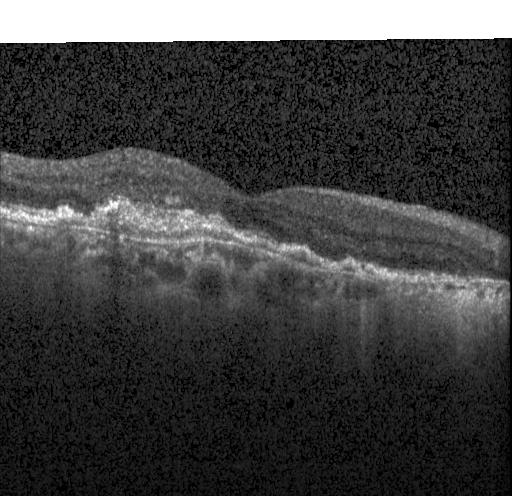 OCT B-scan showing a choroidal neovascular membrane.